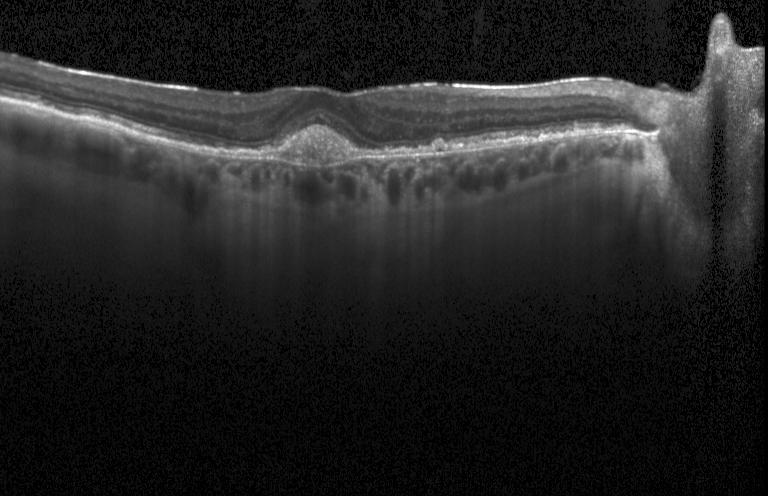
Optical coherence tomography scan · spectral-domain OCT · fovea-centered
Assessment: choroidal neovascularization (CNV).